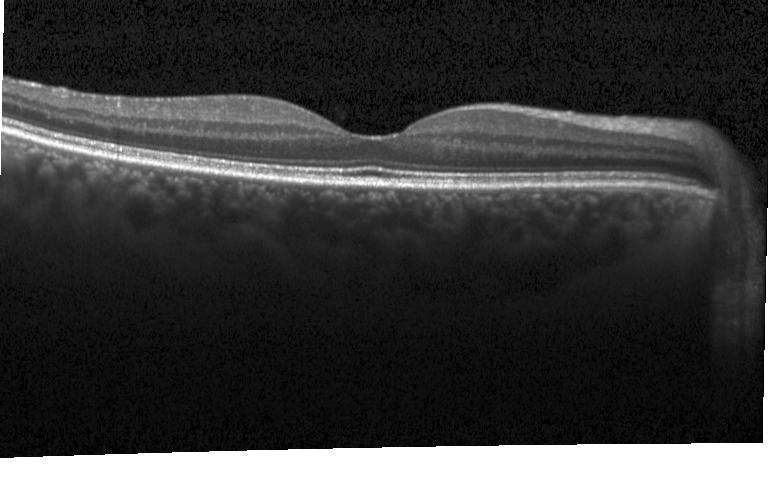
Optical coherence tomography scan
OCT finding: no choroidal neovascularization, diabetic macular edema, or drusen.